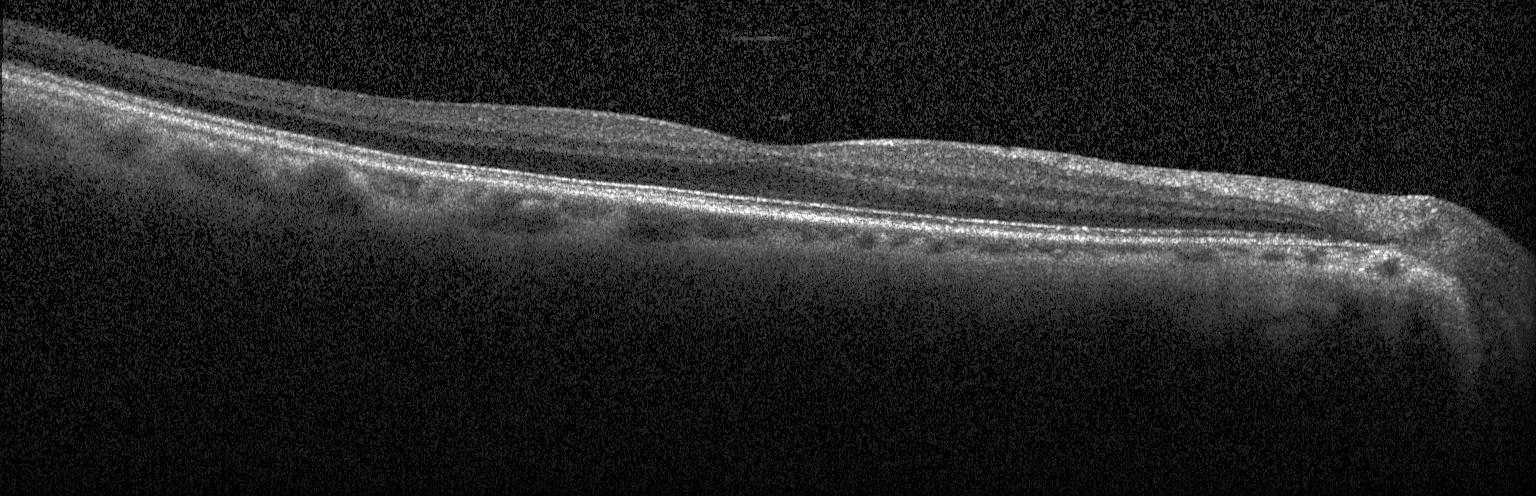
Acquired on a Heidelberg Spectralis, optical coherence tomography B-scan, centered on the fovea, spectral-domain OCT
This B-scan demonstrates no evidence of choroidal neovascularization, diabetic macular edema, or drusen.